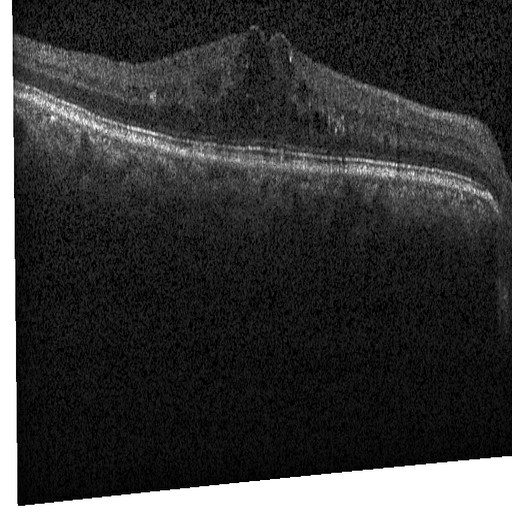
Optical coherence tomography B-scan, fovea-centered, spectral-domain OCT, Heidelberg Spectralis — The scan shows DME.